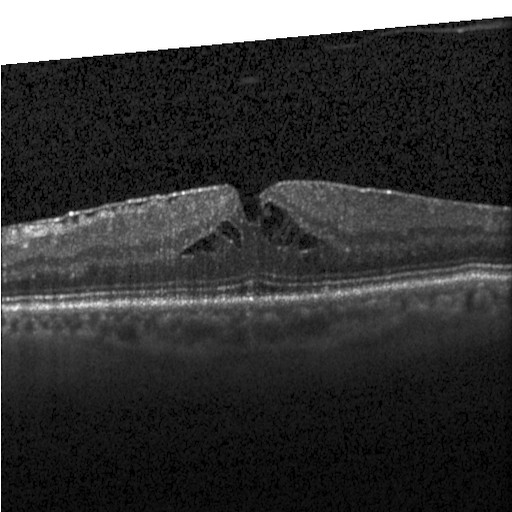 Diabetic macular edema.